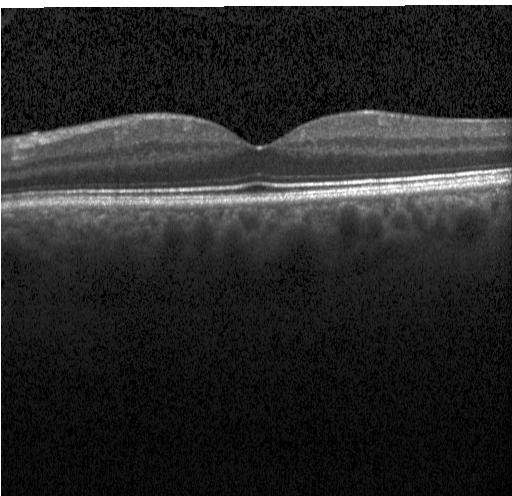

Instrument: Heidelberg Spectralis · OCT B-scan.
Finding: no CNV, DME, or drusen.